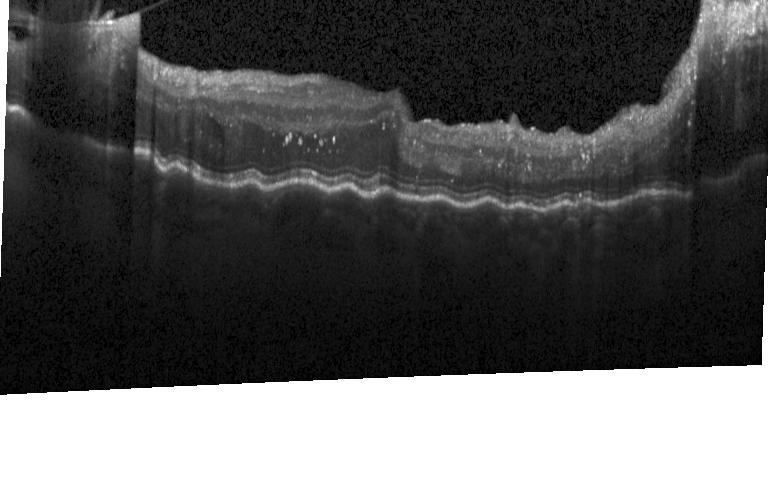

Diagnosis: DME.